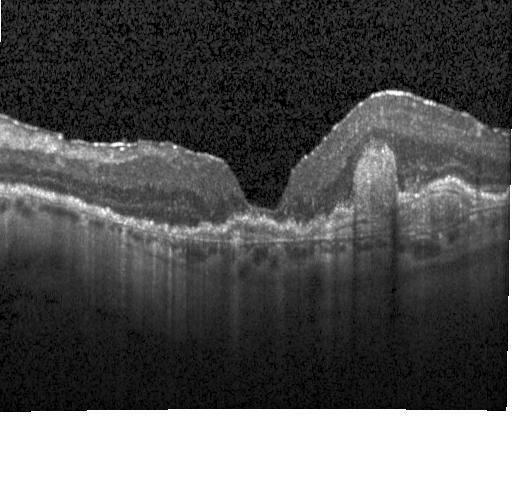
Heidelberg Spectralis, macular scan, optical coherence tomography B-scan, spectral-domain OCT
This B-scan demonstrates CNV.